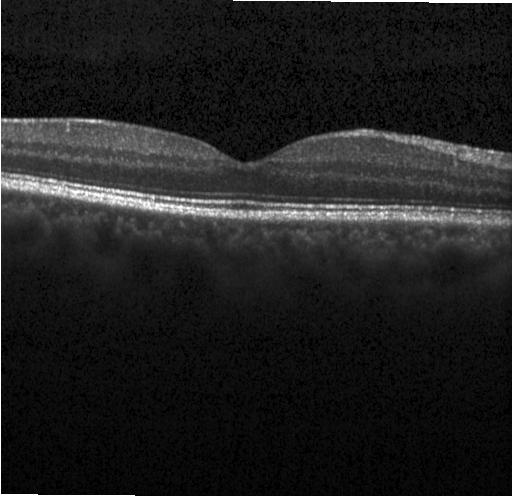

Heidelberg Spectralis; OCT B-scan; centered on the fovea; spectral-domain optical coherence tomography — Finding: neither CNV, DME, nor drusen.